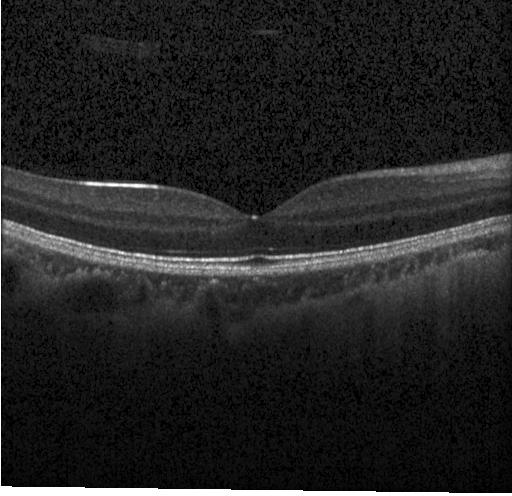

Centered on the fovea · Heidelberg Spectralis · retinal OCT B-scan
Impression: no evidence of CNV, DME, or drusen.